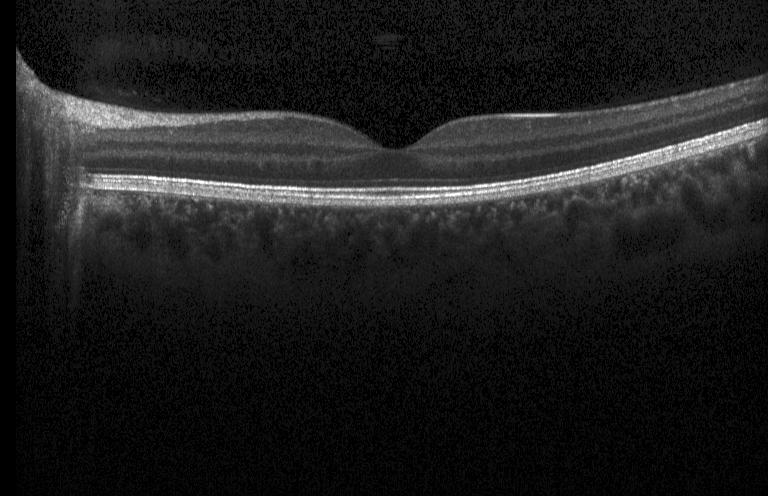
SD-OCT. Optical coherence tomography scan. Assessment: no choroidal neovascularization, no diabetic macular edema, and no drusen.